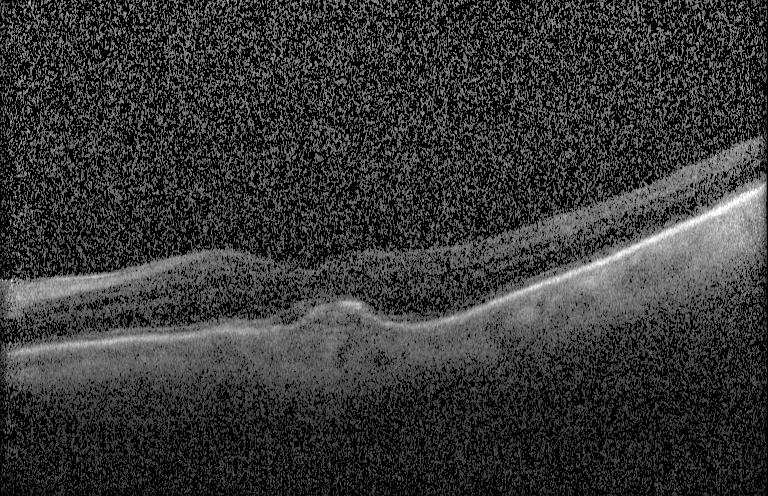

Heidelberg Spectralis, retinal OCT cross-section, fovea-centered, SD-OCT
The scan shows choroidal neovascularization (CNV).